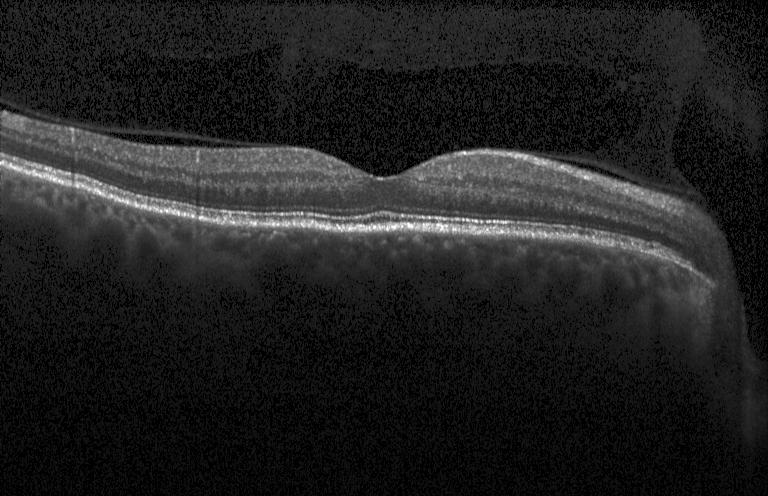 Assessment: no choroidal neovascularization, no diabetic macular edema, and no drusen.